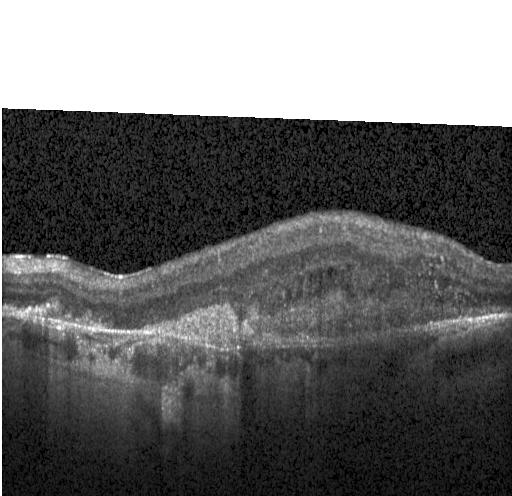
Instrument: Heidelberg Spectralis, OCT line scan, through the macula — The scan shows a choroidal neovascular membrane.